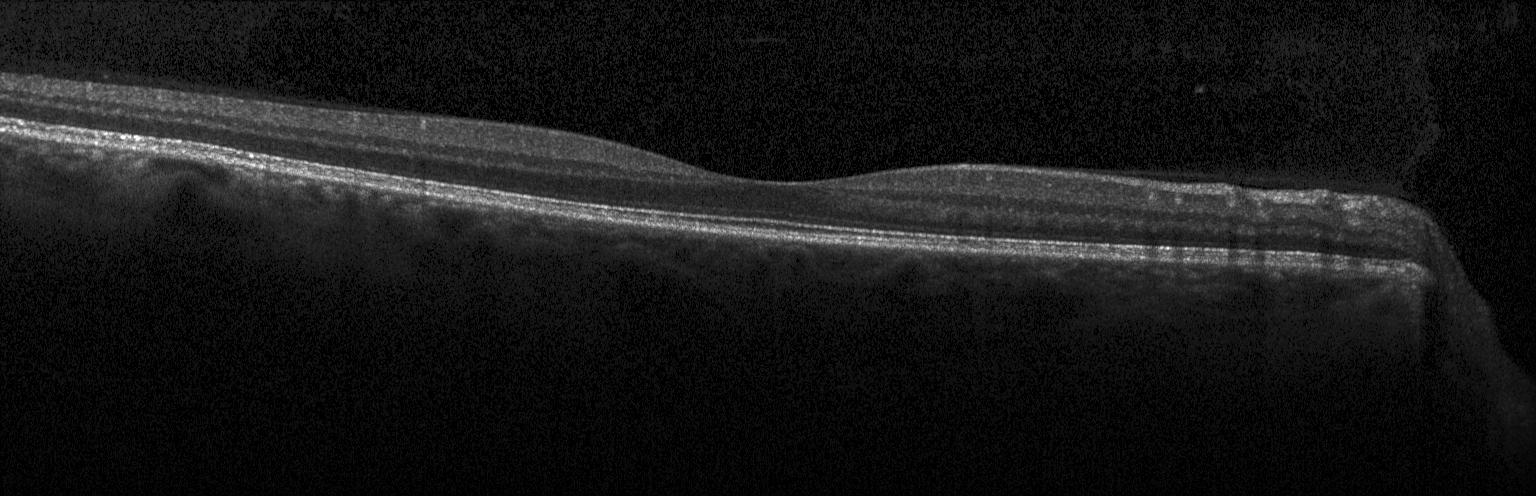
Fovea-centered; retinal OCT cross-section; SD-OCT; instrument: Heidelberg Spectralis
The scan shows no choroidal neovascularization, diabetic macular edema, or drusen.